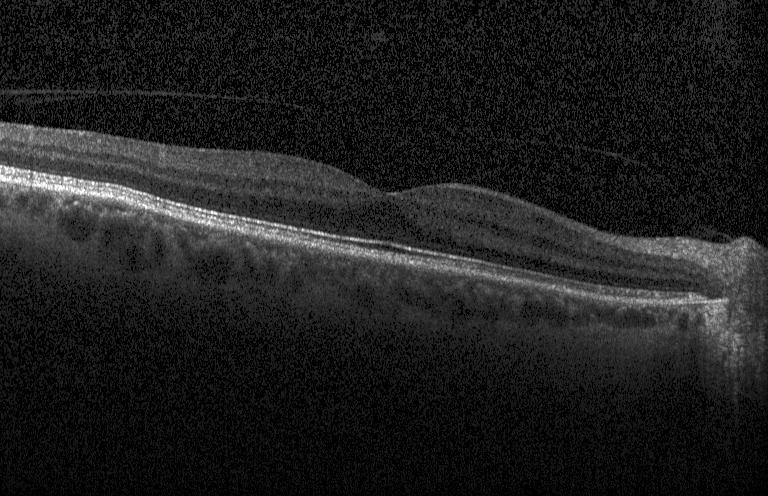

OCT scan showing neither choroidal neovascularization, diabetic macular edema, nor drusen.